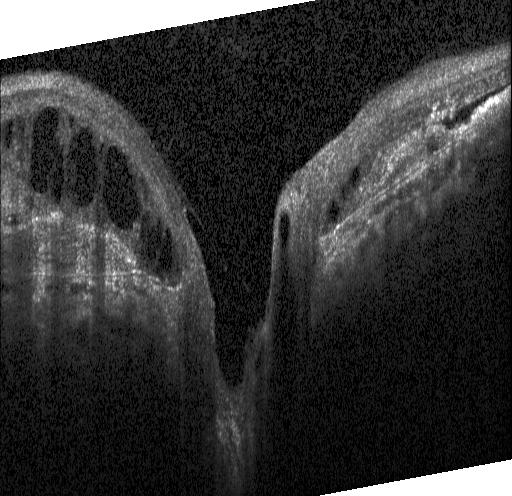
SD-OCT, optical coherence tomography B-scan.
The scan shows choroidal neovascularization.